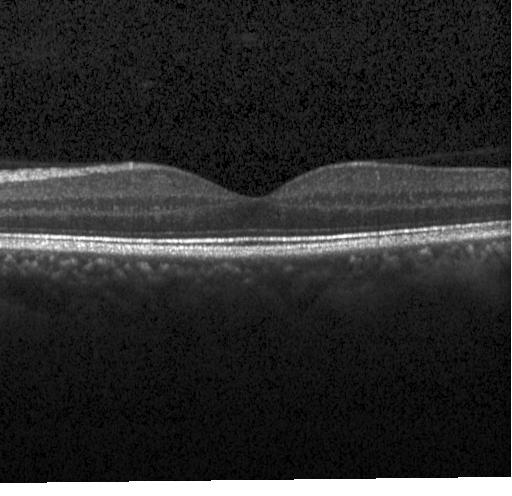

OCT line scan. Through the macula — Impression: no choroidal neovascularization, diabetic macular edema, or drusen.